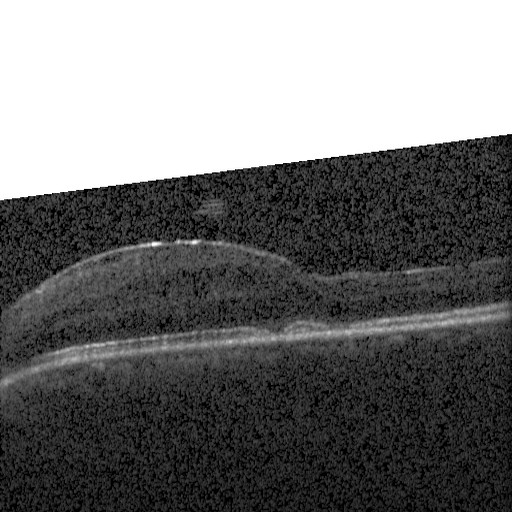

OCT line scan. Diagnosis: diabetic macular edema (DME).